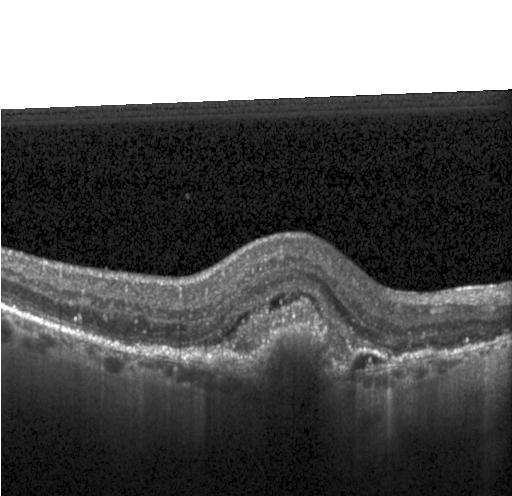
Horizontal scan through the fovea · spectral-domain optical coherence tomography · optical coherence tomography B-scan · Heidelberg Spectralis OCT system. Finding: CNV.